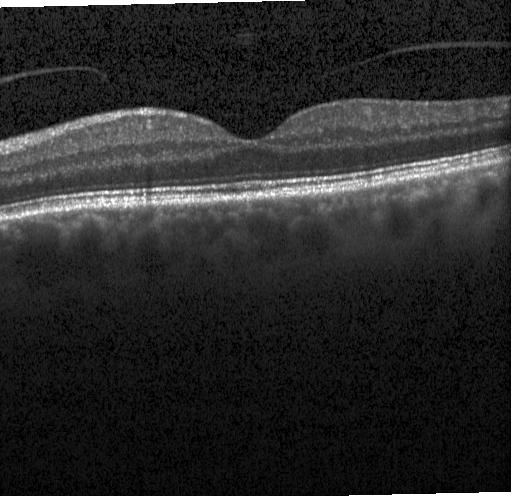 OCT scan showing no choroidal neovascularization, diabetic macular edema, or drusen.